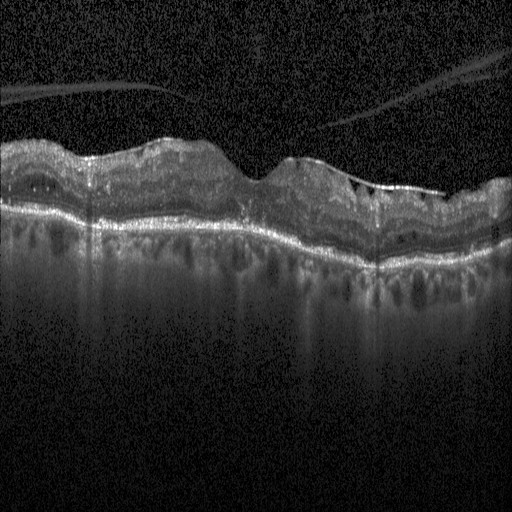
Acquired on a Heidelberg Spectralis. Spectral-domain optical coherence tomography. OCT B-scan. Fovea-centered. Dx: DME.